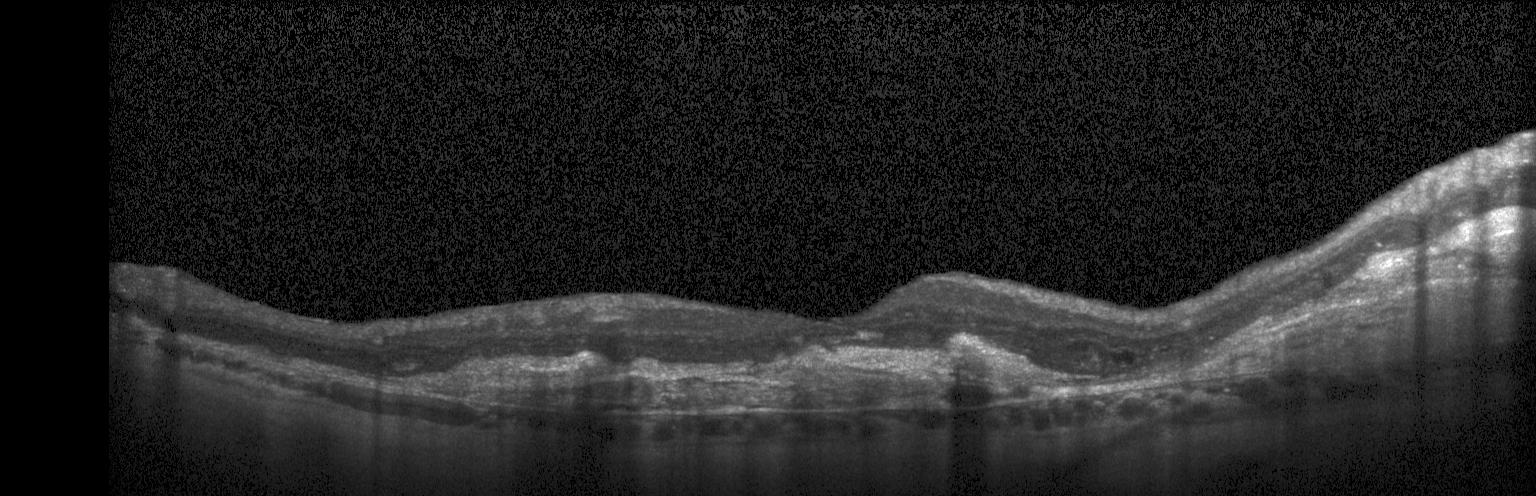 OCT B-scan; instrument: Heidelberg Spectralis
Impression: choroidal neovascularization (CNV).